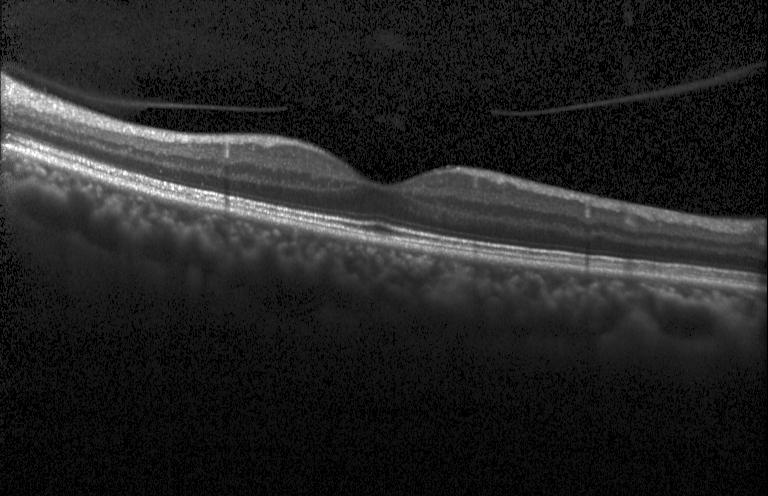

Dx: no evidence of CNV, DME, or drusen.